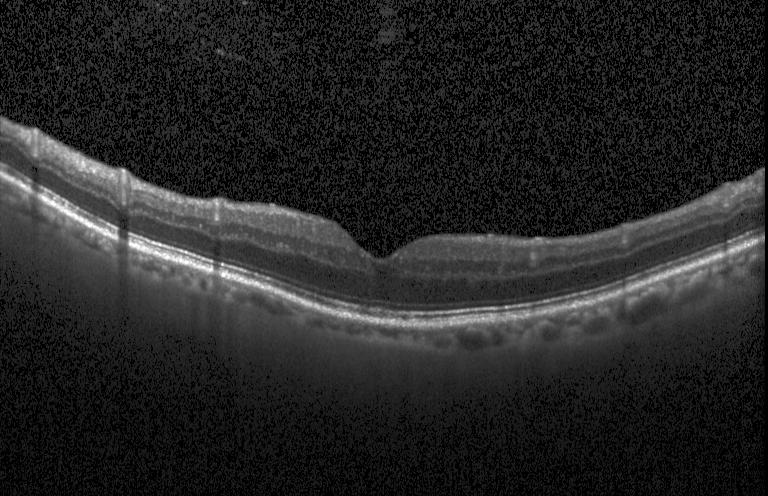

Macular OCT demonstrating neither CNV, DME, nor drusen.